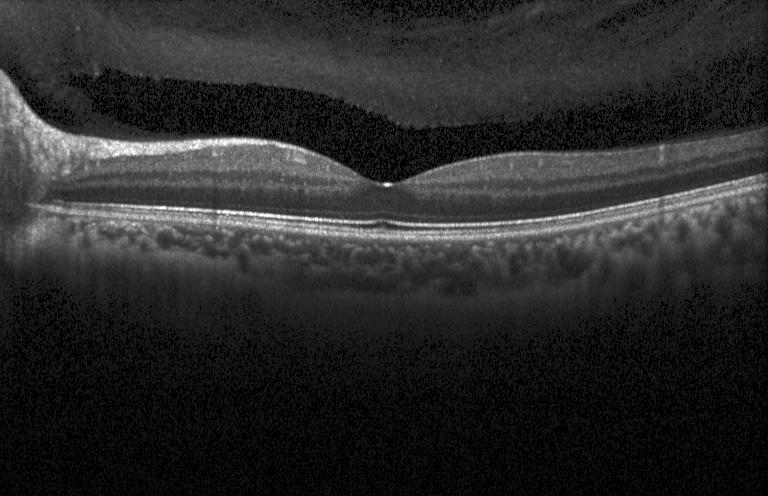

Centered on the fovea · SD-OCT · Heidelberg Spectralis · OCT B-scan. Finding: neither choroidal neovascularization, diabetic macular edema, nor drusen.